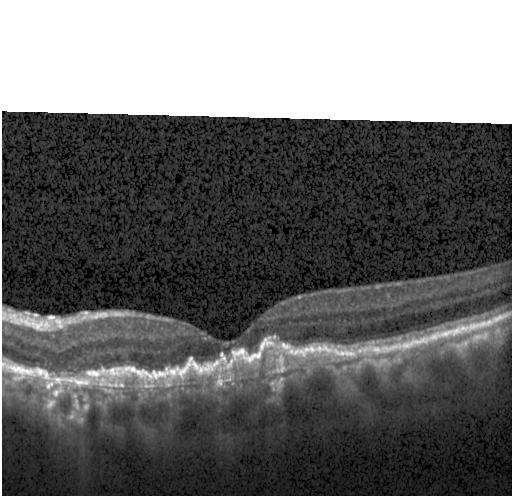

Acquired on a Heidelberg Spectralis; SD-OCT; retinal OCT cross-section; fovea-centered — OCT finding: a choroidal neovascular membrane.